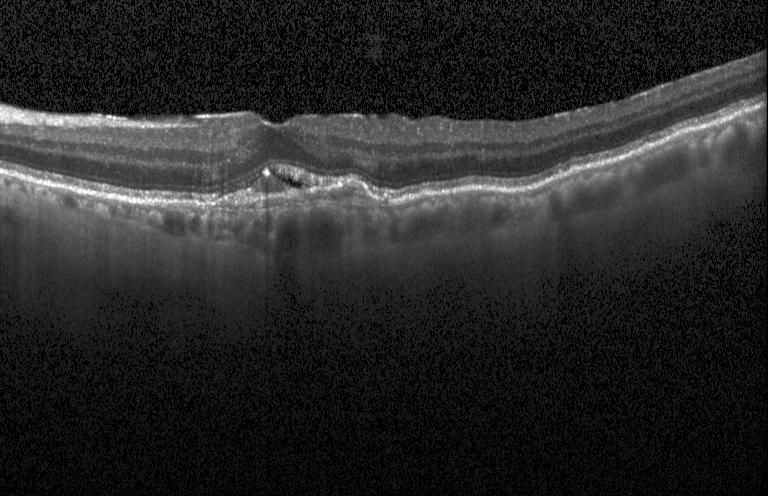 Heidelberg Spectralis OCT system · horizontal scan through the fovea · OCT line scan · spectral-domain OCT. Finding: choroidal neovascularization.